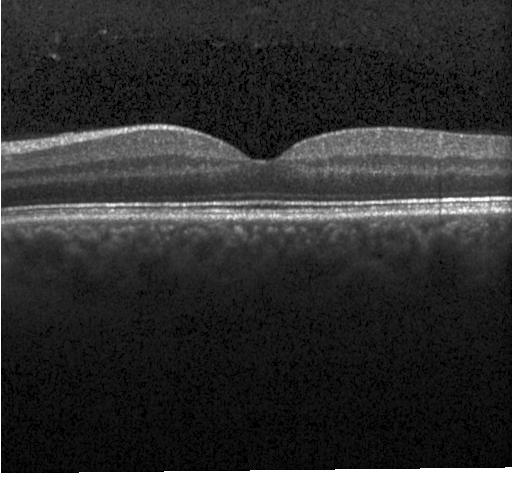
OCT finding: no CNV, no DME, and no drusen.